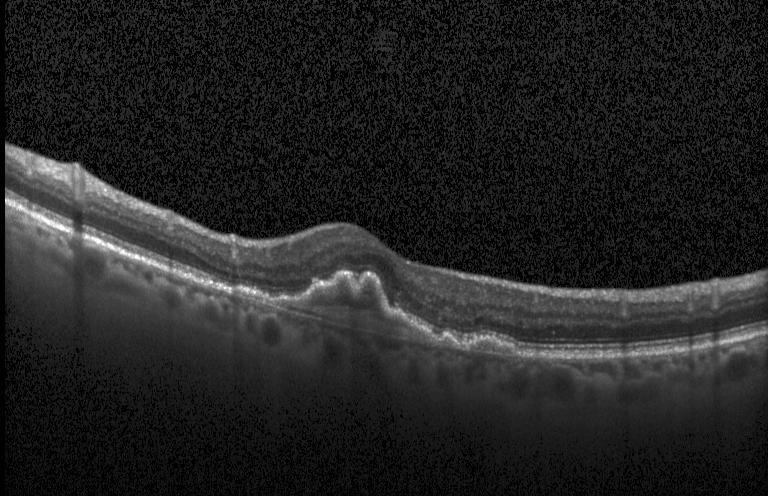 OCT scan showing a choroidal neovascular membrane.